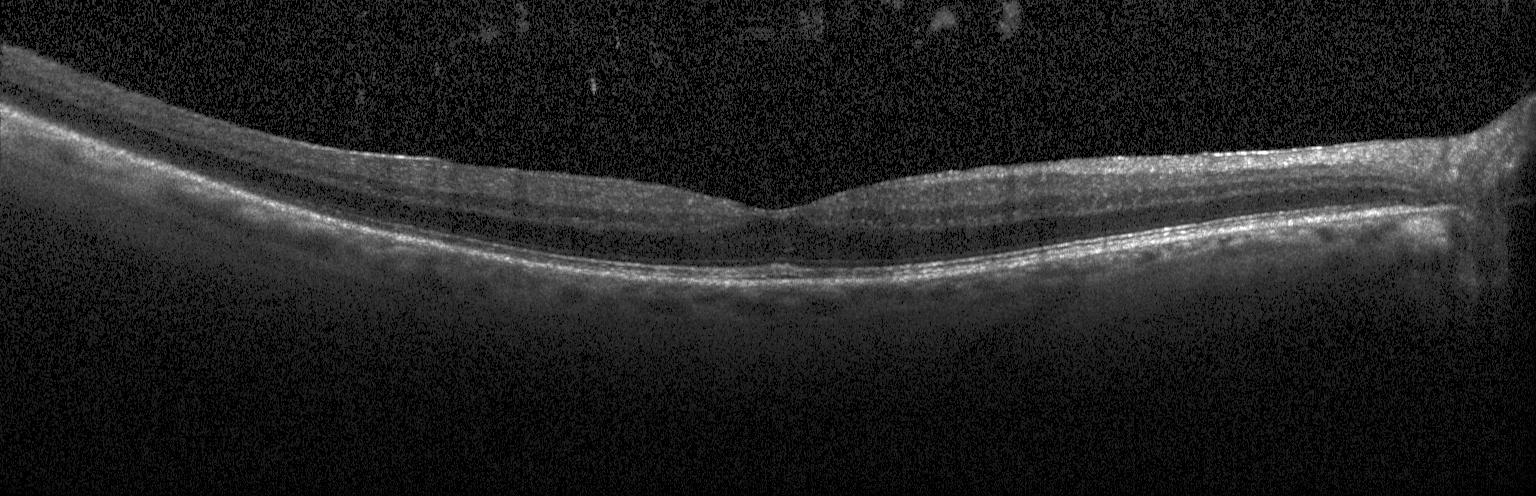
Finding: neither CNV, DME, nor drusen.